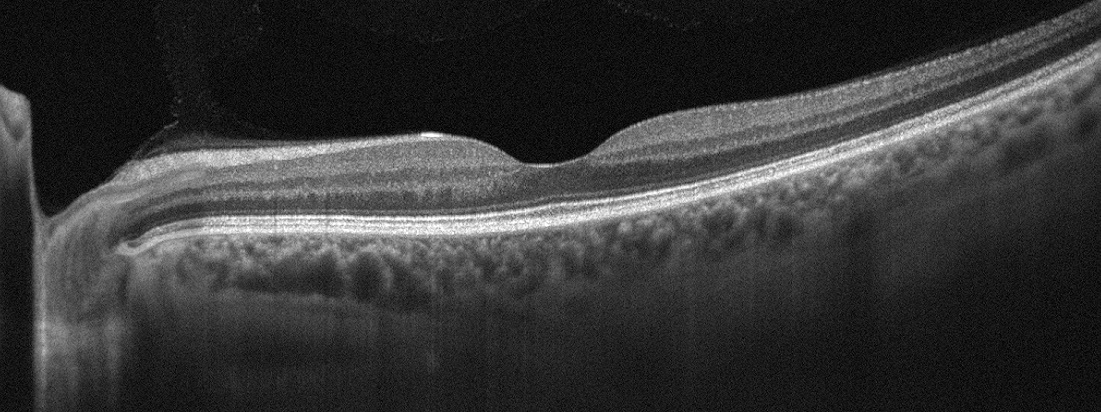
Diagnosis: no evidence of AMD, DME, ERM, RAO, RVO, or VID.